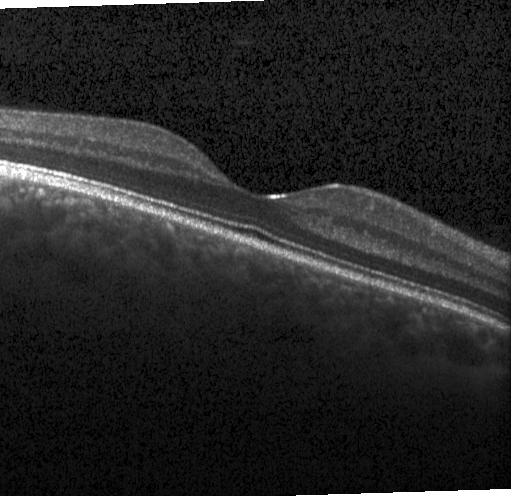 Finding: neither choroidal neovascularization, diabetic macular edema, nor drusen.